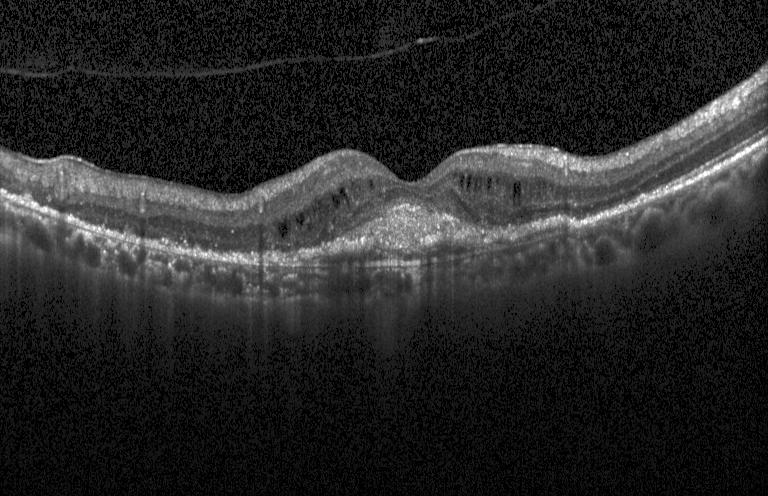 Finding: CNV.